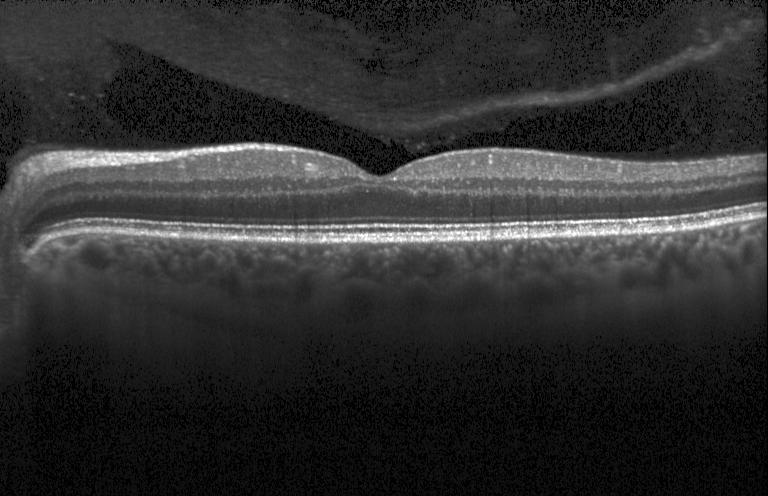
Instrument: Heidelberg Spectralis; SD-OCT; optical coherence tomography scan; macular scan.
Dx: no choroidal neovascularization, diabetic macular edema, or drusen.